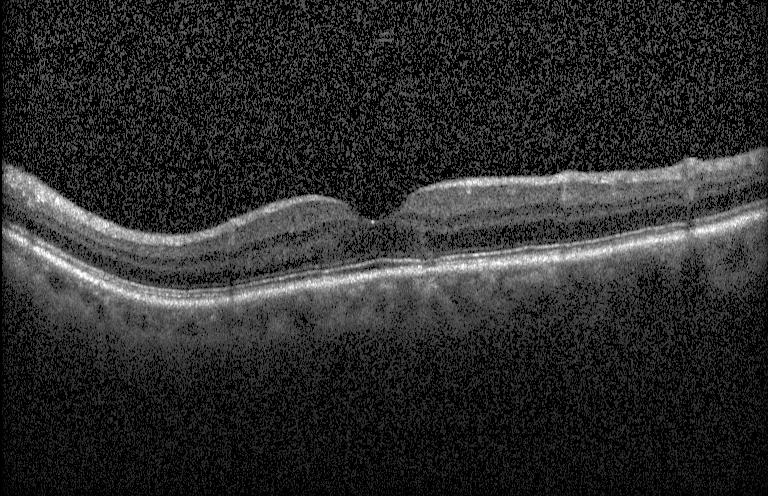
Optical coherence tomography scan. Diagnosis: neither choroidal neovascularization, diabetic macular edema, nor drusen.